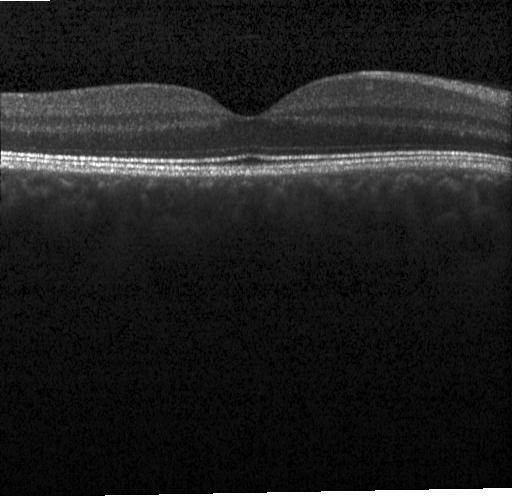
Retinal OCT B-scan, spectral-domain optical coherence tomography, horizontal scan through the fovea
Macular OCT: no choroidal neovascularization, diabetic macular edema, or drusen.